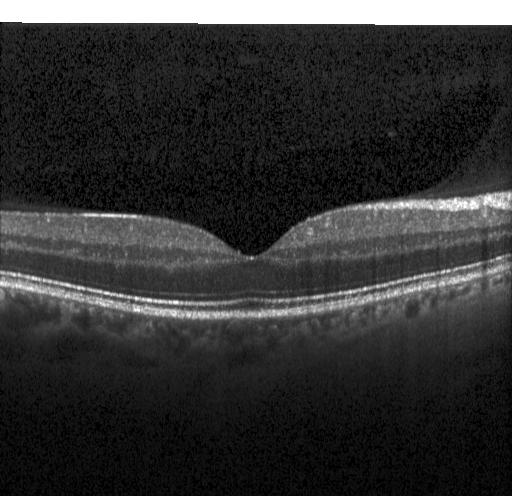 Impression: no choroidal neovascularization, diabetic macular edema, or drusen.